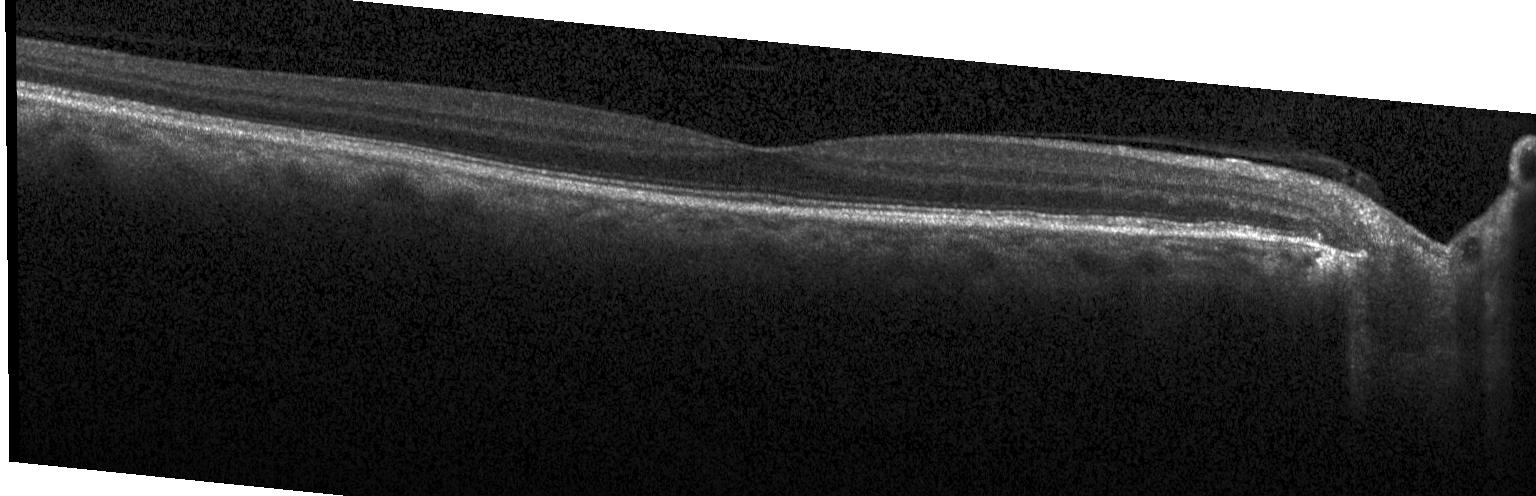

Acquired on a Heidelberg Spectralis. Spectral-domain optical coherence tomography. Optical coherence tomography scan. Centered on the fovea — Diagnosis: no choroidal neovascularization, diabetic macular edema, or drusen.